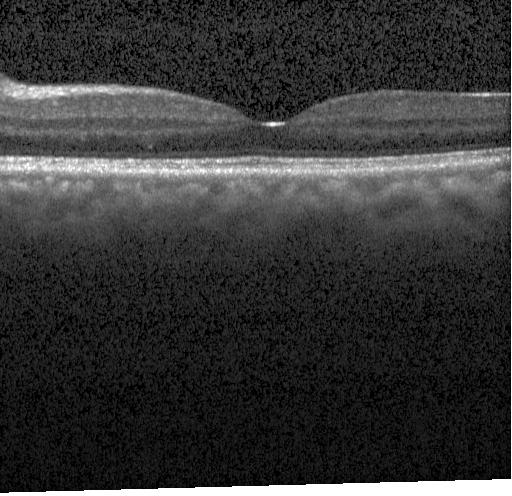 Impression: no choroidal neovascularization, no diabetic macular edema, and no drusen.